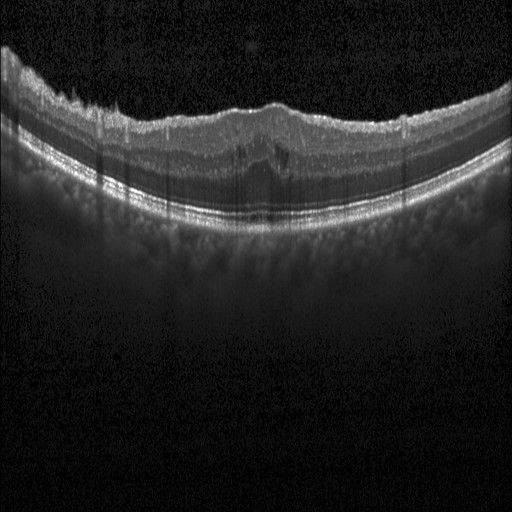
Optical coherence tomography B-scan, spectral-domain optical coherence tomography — Assessment: DME.